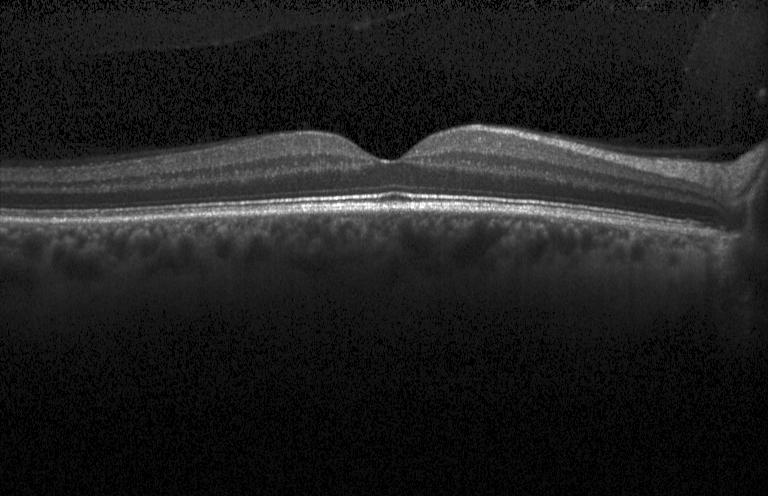 Assessment: no choroidal neovascularization, no diabetic macular edema, and no drusen.